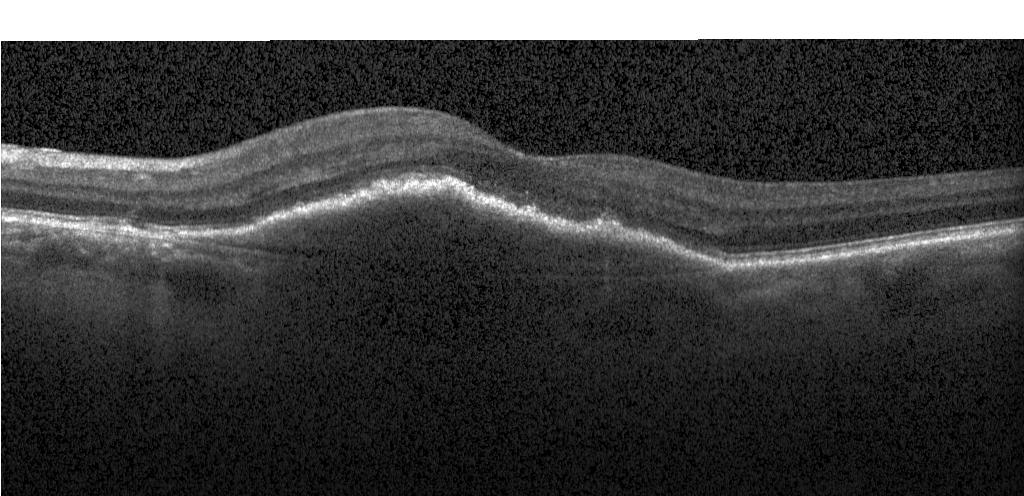

Optical coherence tomography scan. Fovea-centered
Diagnosis: a choroidal neovascular membrane.